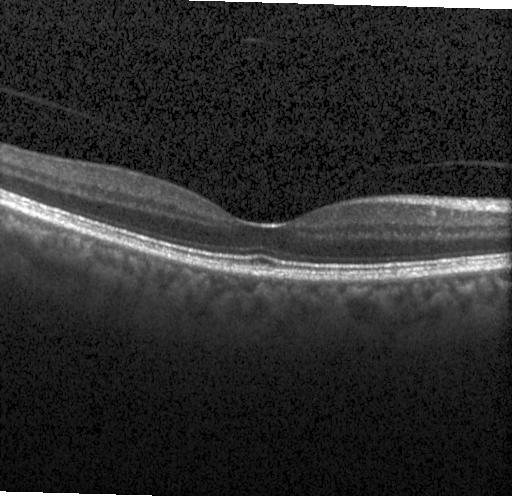
Spectral-domain OCT, fovea-centered, OCT B-scan
This B-scan demonstrates neither choroidal neovascularization, diabetic macular edema, nor drusen.